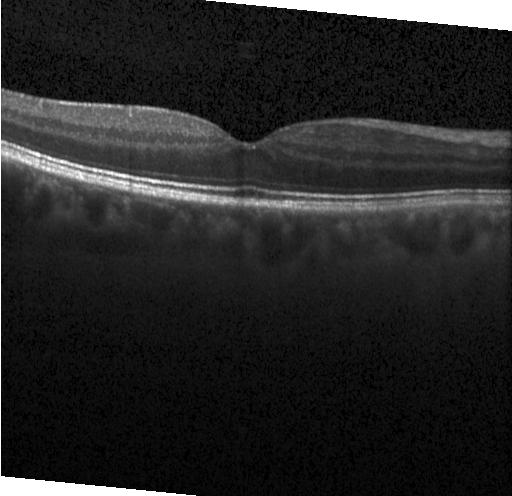

Fovea-centered, OCT line scan, instrument: Heidelberg Spectralis.
Diagnosis: neither choroidal neovascularization, diabetic macular edema, nor drusen.